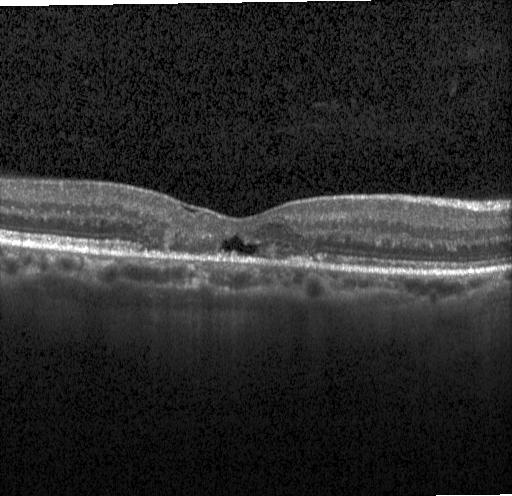 A choroidal neovascular membrane.